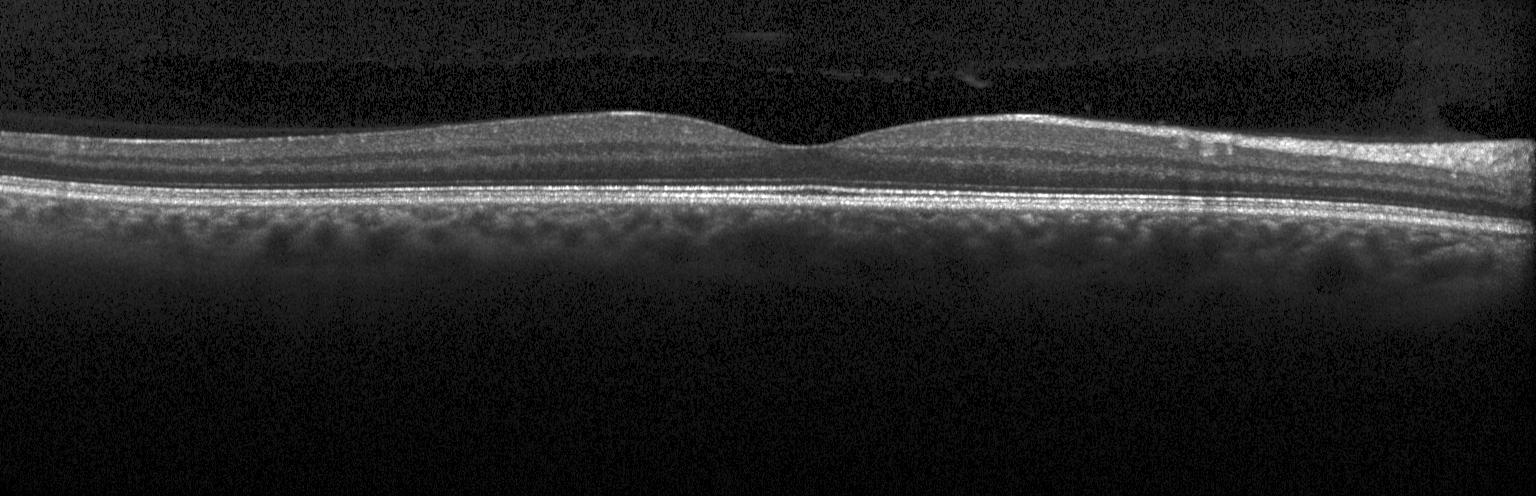 Optical coherence tomography B-scan · instrument: Heidelberg Spectralis · spectral-domain optical coherence tomography · through the macula — Diagnosis: neither choroidal neovascularization, diabetic macular edema, nor drusen.